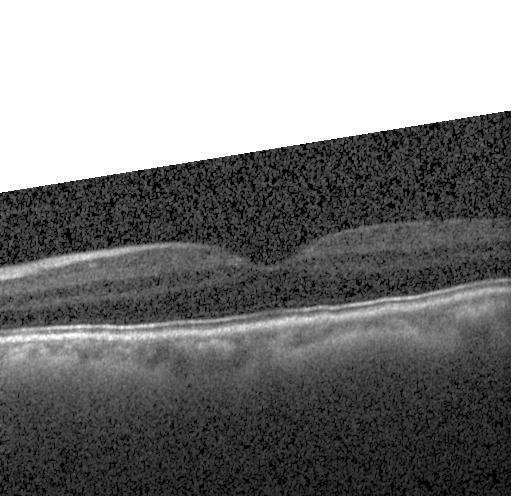 Retinal OCT B-scan, SD-OCT.
Finding: no evidence of choroidal neovascularization, diabetic macular edema, or drusen.